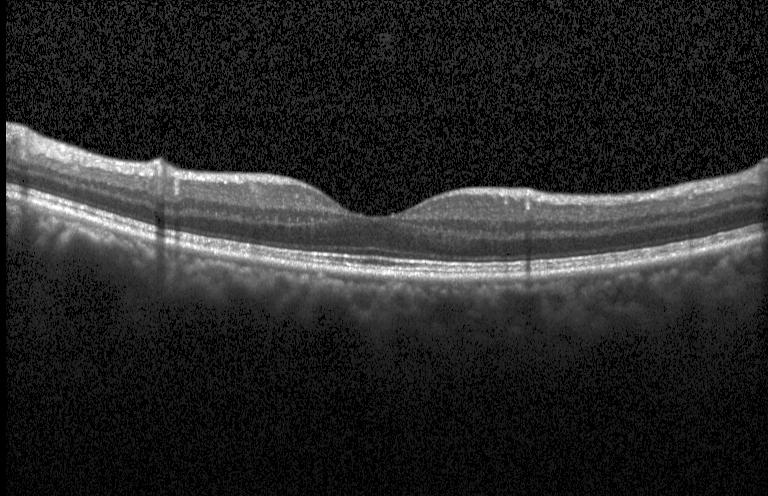 Optical coherence tomography scan
The scan shows no choroidal neovascularization, diabetic macular edema, or drusen.